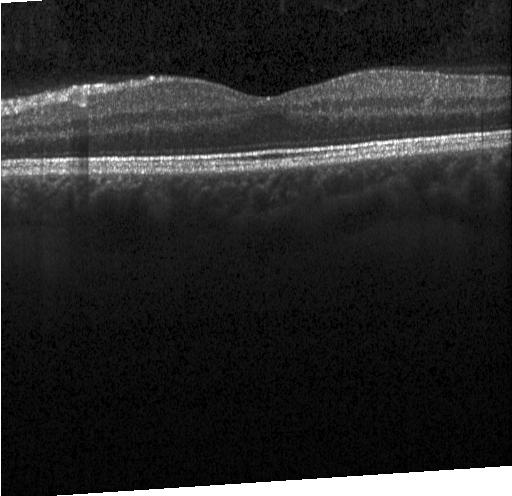 Spectral-domain optical coherence tomography · OCT line scan.
Impression: no choroidal neovascularization, diabetic macular edema, or drusen.